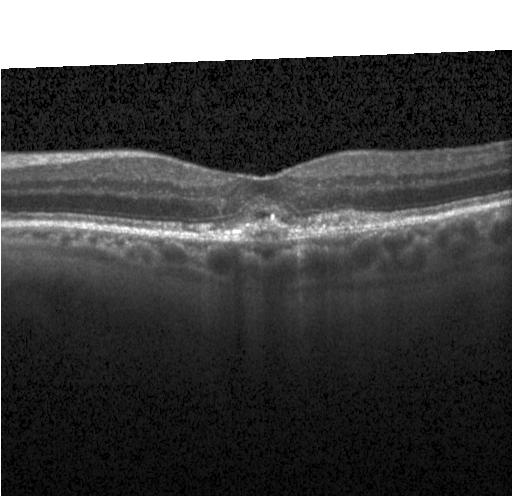

OCT B-scan; through the macula; spectral-domain optical coherence tomography
Diagnosis: a choroidal neovascular membrane.